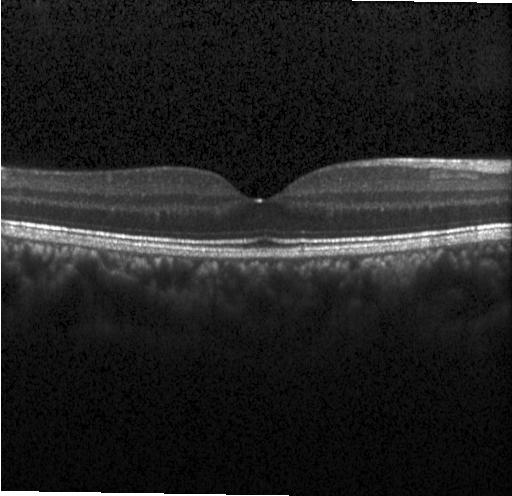 OCT scan showing neither choroidal neovascularization, diabetic macular edema, nor drusen.